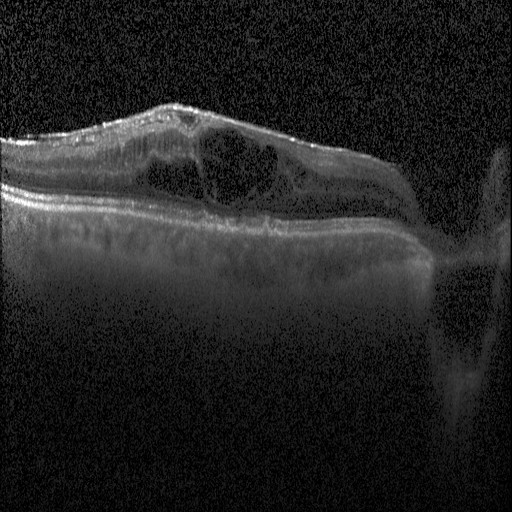 Finding: DME.